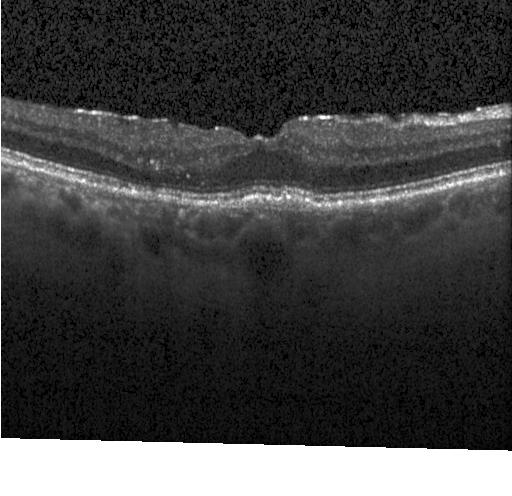 Spectral-domain optical coherence tomography; OCT B-scan. Finding: CNV.